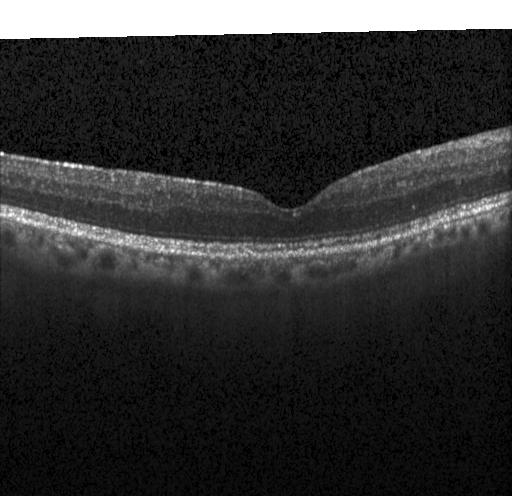 OCT line scan — No choroidal neovascularization, diabetic macular edema, or drusen.